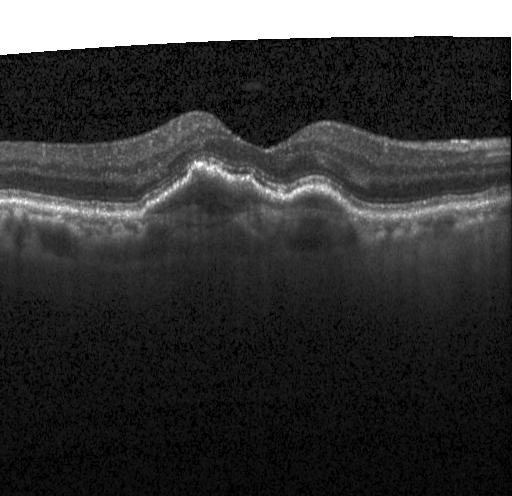 Optical coherence tomography B-scan.
Dx: a choroidal neovascular membrane.